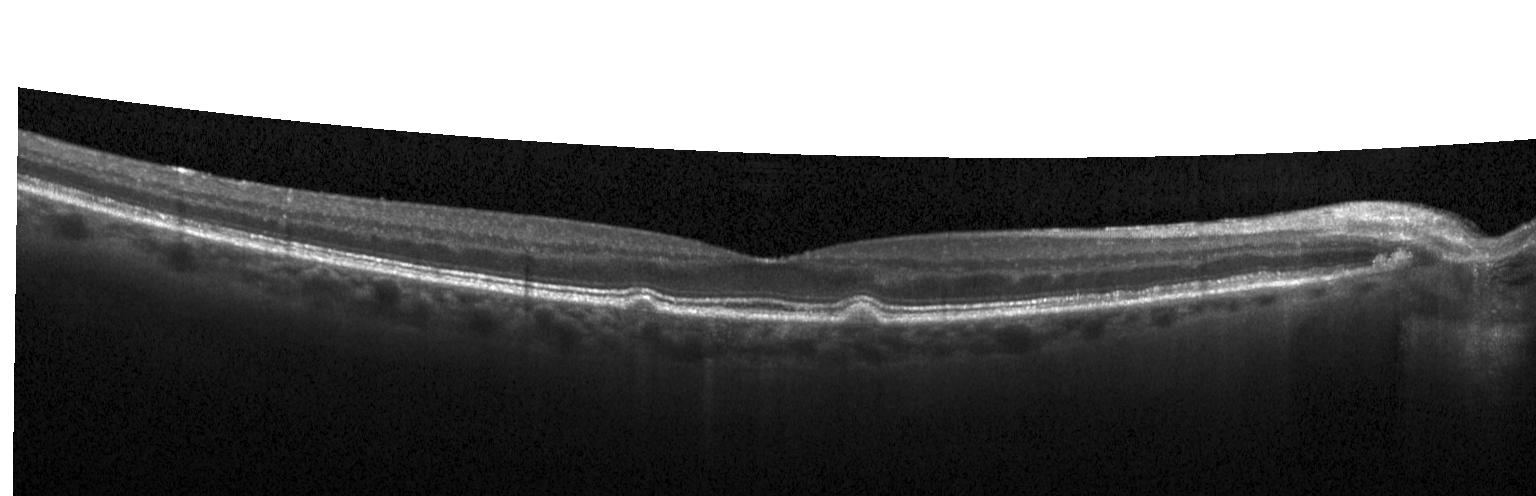 Heidelberg Spectralis, retinal OCT B-scan
This B-scan demonstrates sub-RPE drusenoid deposits.